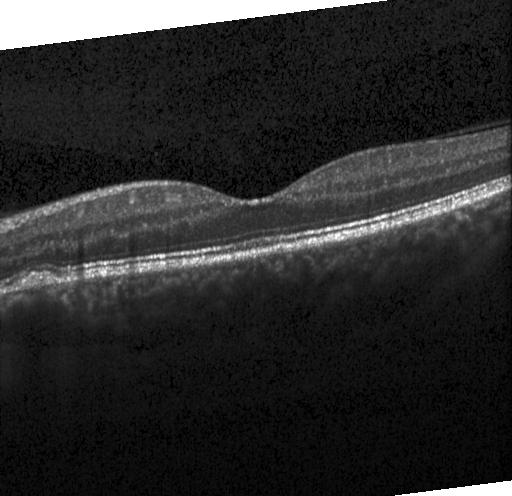

Retinal OCT B-scan; horizontal scan through the fovea; acquired on a Heidelberg Spectralis; spectral-domain OCT.
Macular OCT: sub-RPE drusenoid deposits.